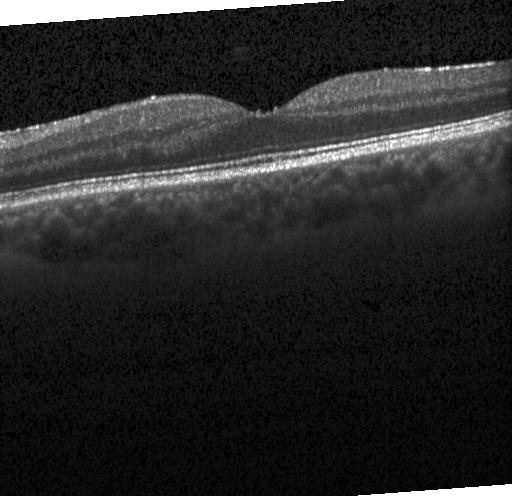 Spectral-domain optical coherence tomography; optical coherence tomography scan; instrument: Heidelberg Spectralis.
Finding: neither CNV, DME, nor drusen.